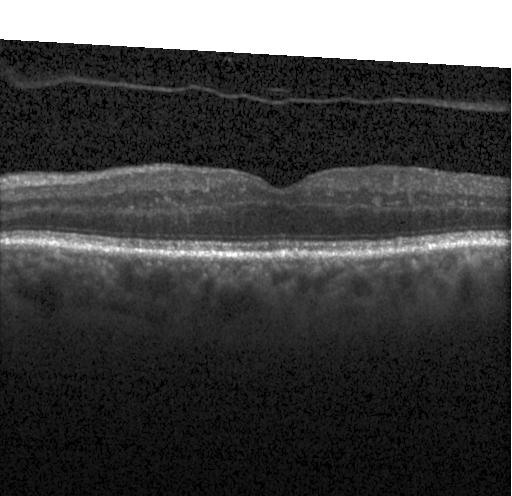
Finding: no evidence of choroidal neovascularization, diabetic macular edema, or drusen.